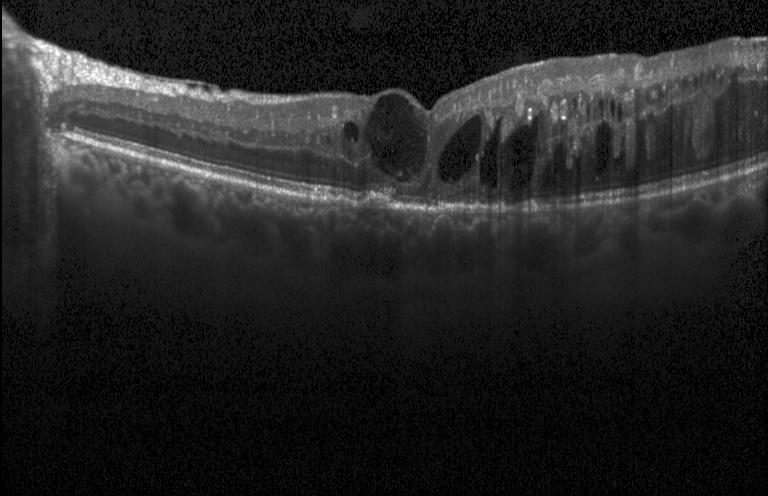 Heidelberg Spectralis OCT system, horizontal scan through the fovea, spectral-domain OCT, retinal OCT B-scan.
OCT finding: diabetic macular edema (DME).